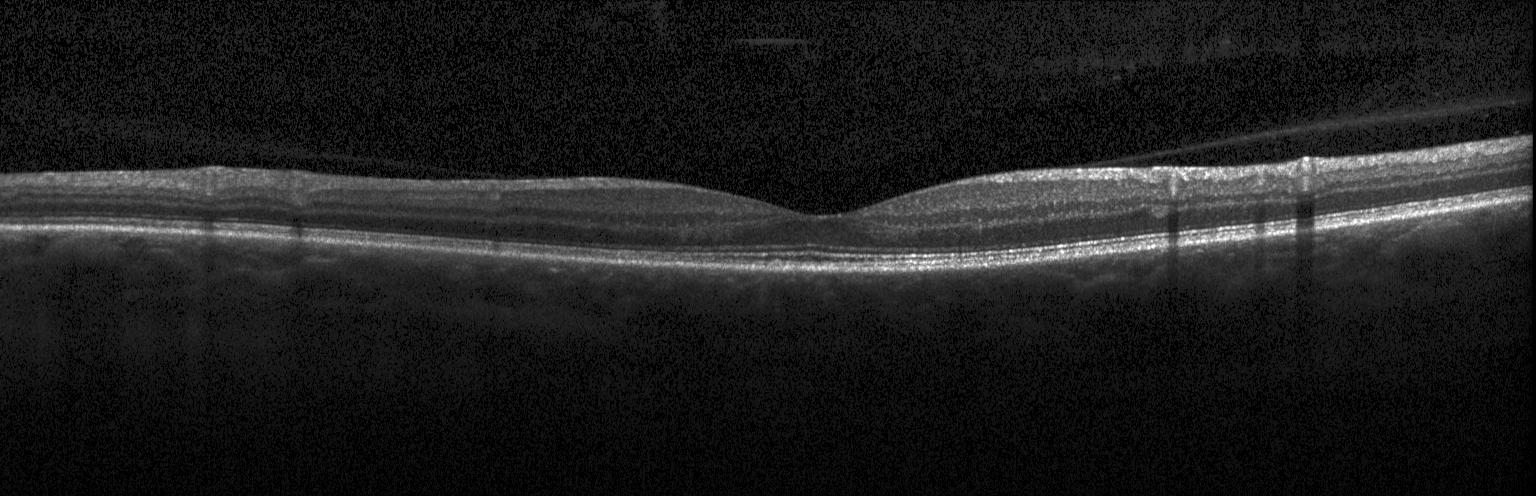 Macular OCT demonstrating neither choroidal neovascularization, diabetic macular edema, nor drusen.